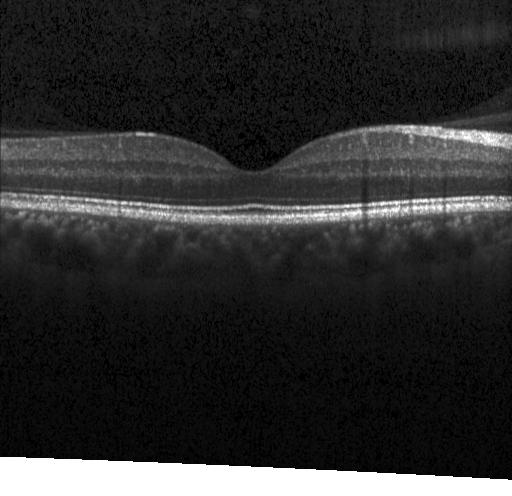
OCT scan showing no evidence of CNV, DME, or drusen.